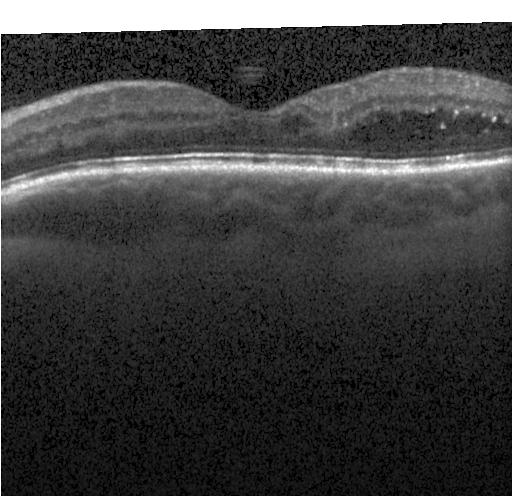
Heidelberg Spectralis; fovea-centered; retinal OCT cross-section
This B-scan demonstrates DME.